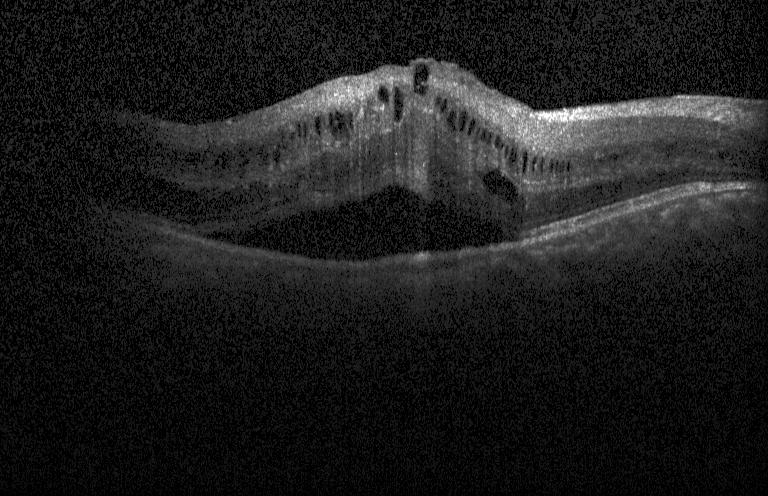

Heidelberg Spectralis. OCT B-scan
OCT finding: diabetic macular edema (DME).